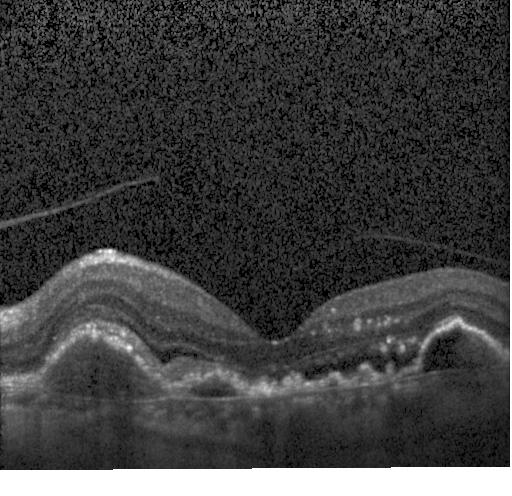
Assessment: choroidal neovascularization.